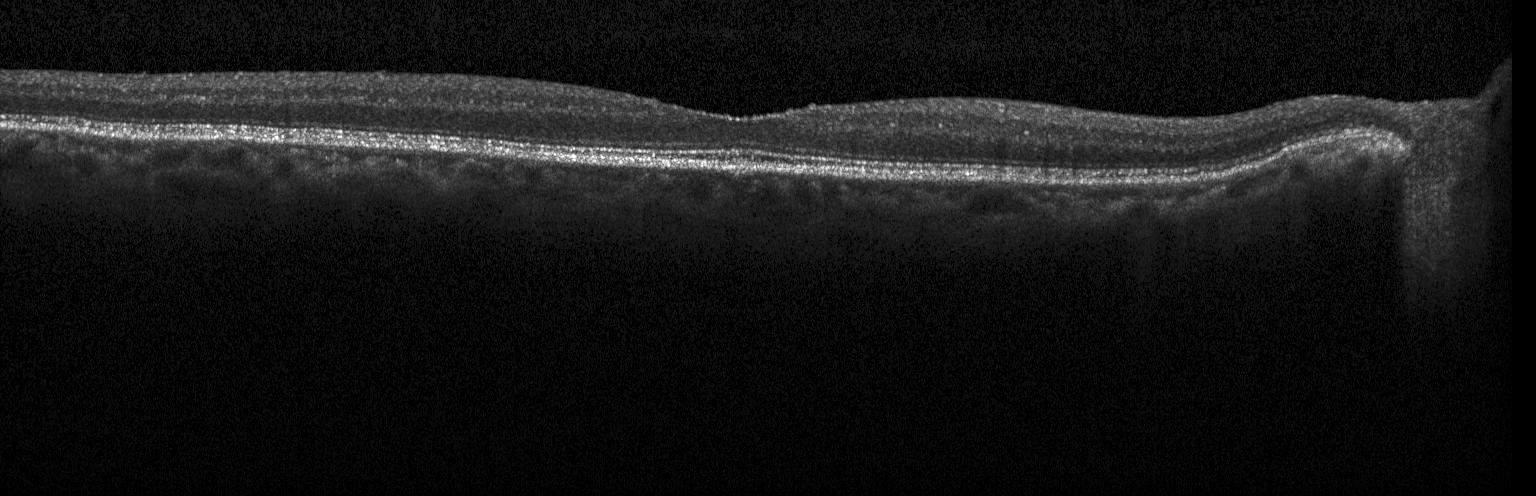

Impression: no evidence of choroidal neovascularization, diabetic macular edema, or drusen.